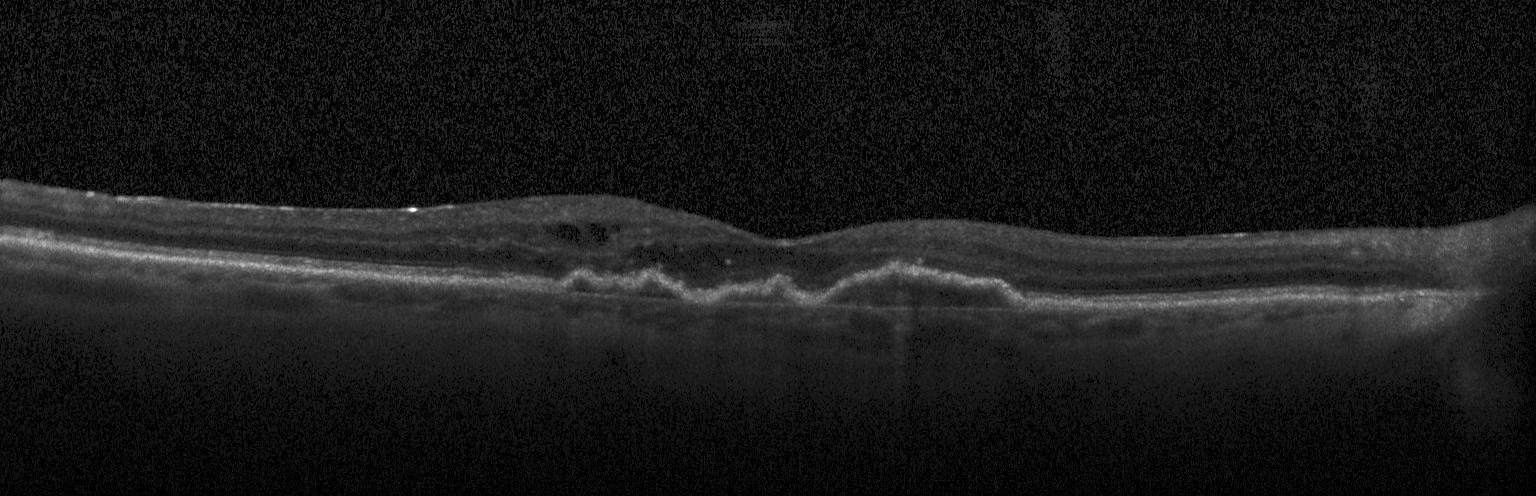
Impression: CNV.